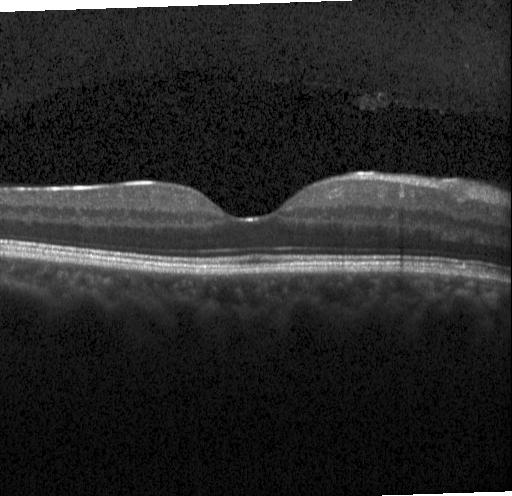

Macular OCT demonstrating no choroidal neovascularization, diabetic macular edema, or drusen.